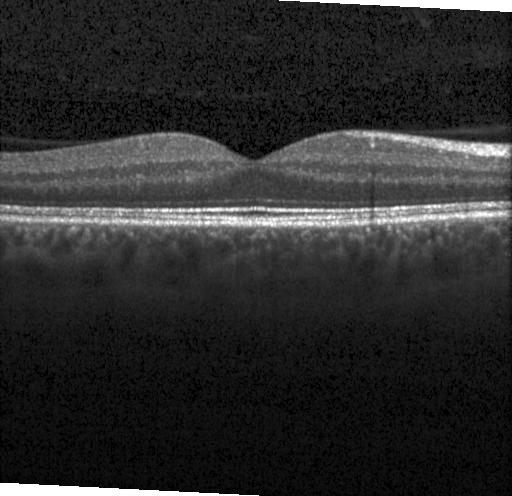
Instrument: Heidelberg Spectralis · retinal OCT cross-section · SD-OCT.
Diagnosis: neither CNV, DME, nor drusen.